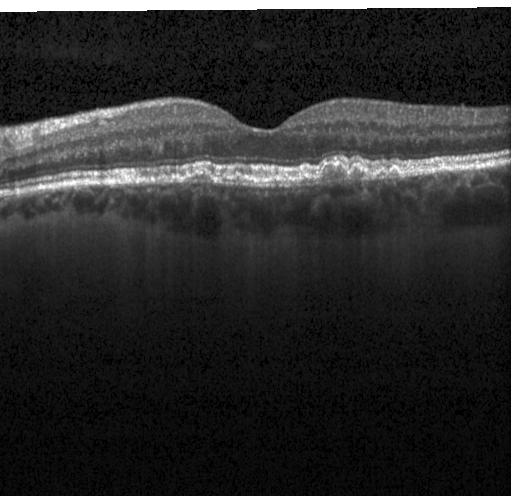 Impression: sub-RPE drusenoid deposits.